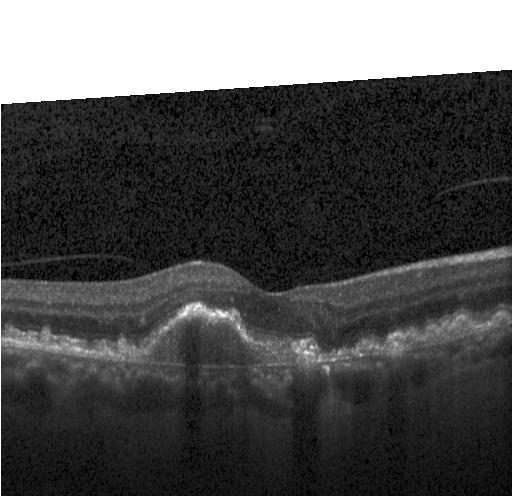
Retinal OCT B-scan.
Impression: CNV.